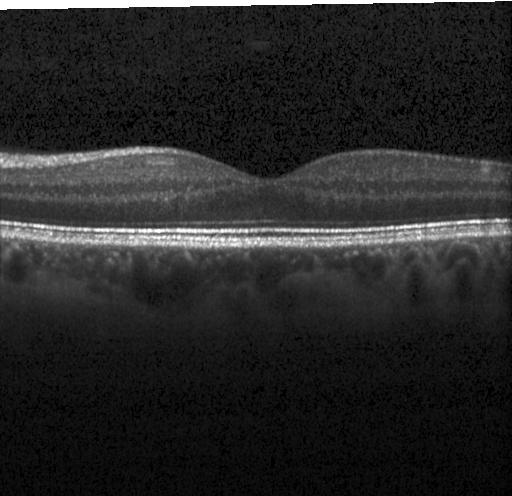

Spectral-domain OCT. Through the macula. Retinal OCT cross-section
Impression: no choroidal neovascularization, diabetic macular edema, or drusen.